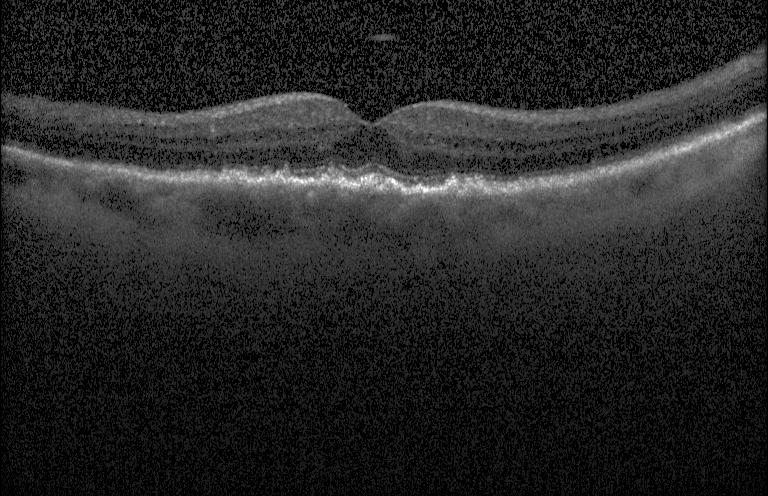 Drusen.